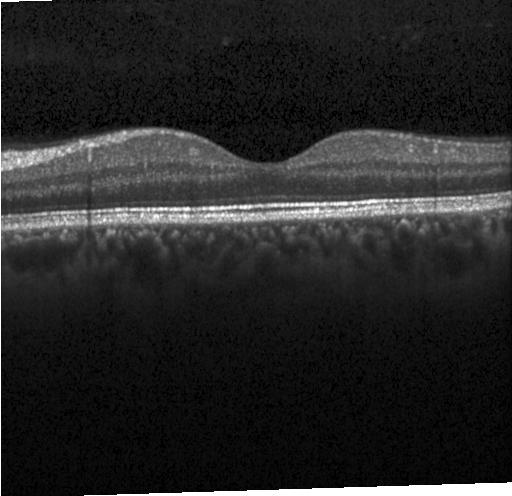

Instrument: Heidelberg Spectralis; spectral-domain optical coherence tomography; fovea-centered; retinal OCT cross-section
Dx: no evidence of choroidal neovascularization, diabetic macular edema, or drusen.